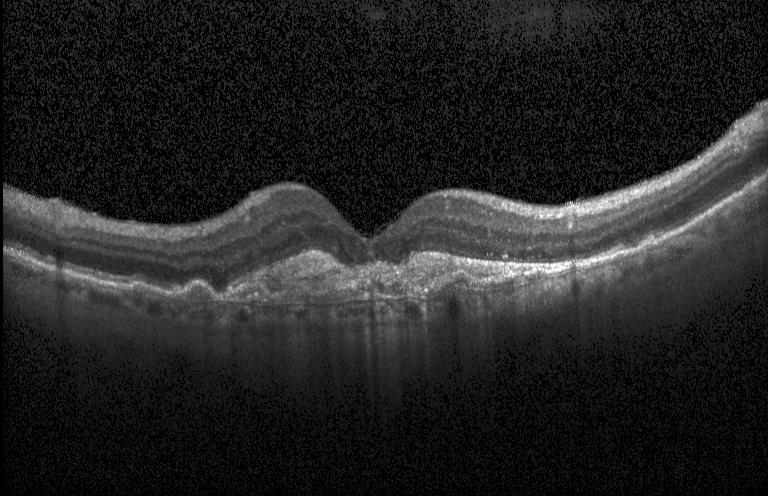
Through the macula, Heidelberg Spectralis, spectral-domain optical coherence tomography, retinal OCT B-scan. Impression: choroidal neovascularization (CNV).